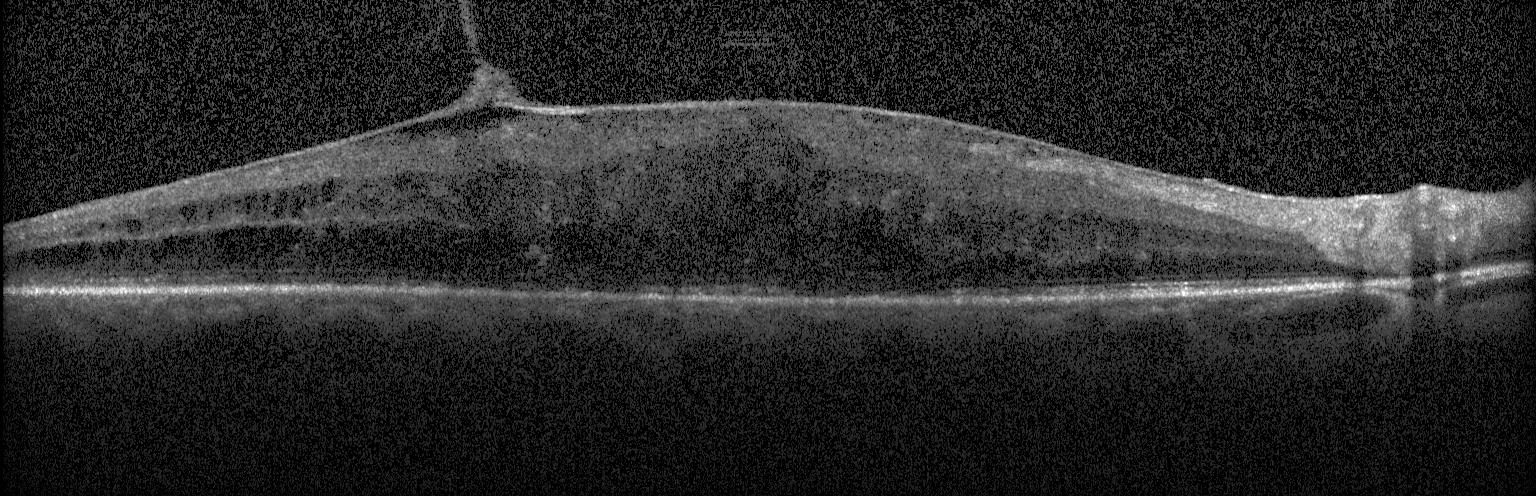 Retinal OCT cross-section · SD-OCT · horizontal scan through the fovea — Finding: DME.